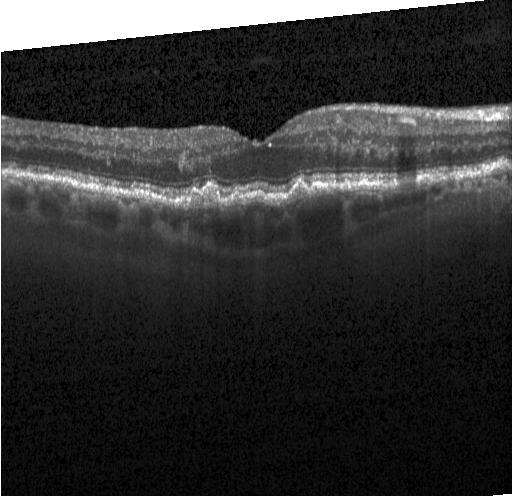
Centered on the fovea; retinal OCT B-scan
Assessment: drusen.